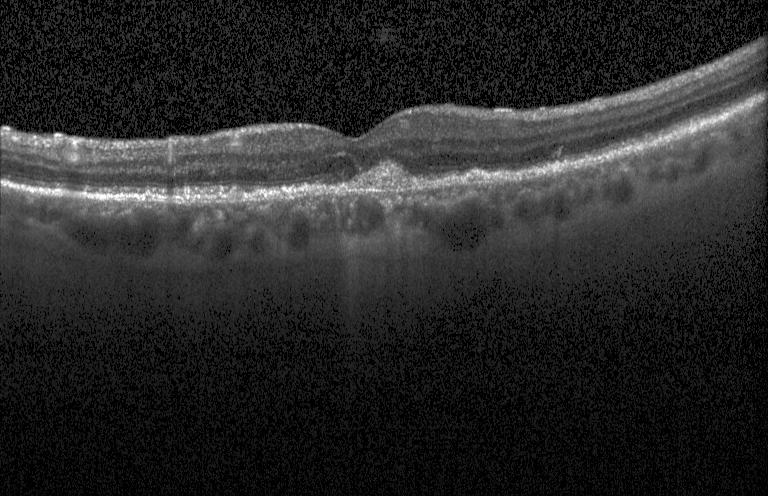

Optical coherence tomography B-scan · Heidelberg Spectralis — Assessment: a choroidal neovascular membrane.